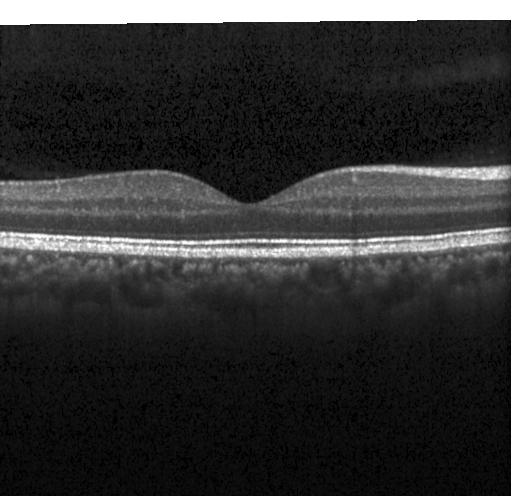

Fovea-centered. OCT line scan. Dx: neither choroidal neovascularization, diabetic macular edema, nor drusen.